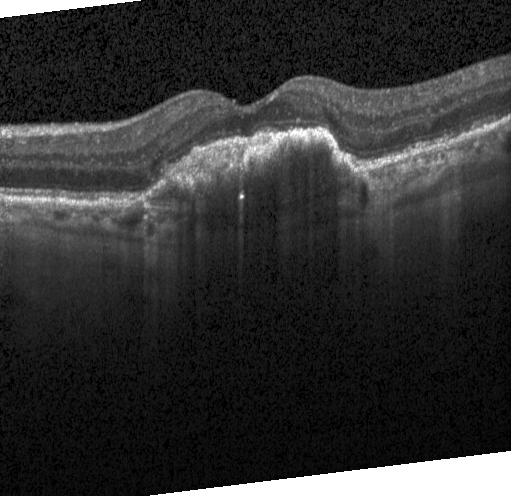
Centered on the fovea. SD-OCT. OCT B-scan.
Macular OCT: CNV.